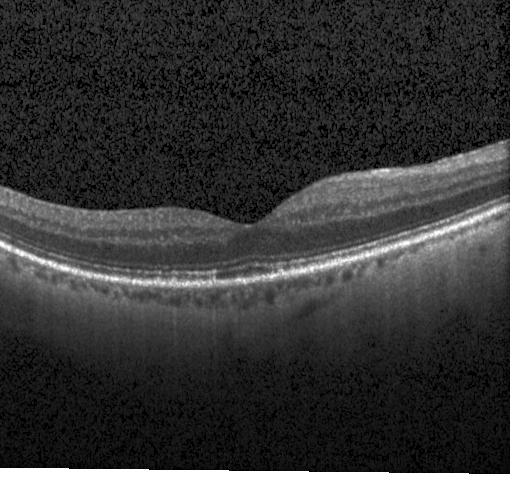 Retinal OCT B-scan. The scan shows no choroidal neovascularization, diabetic macular edema, or drusen.